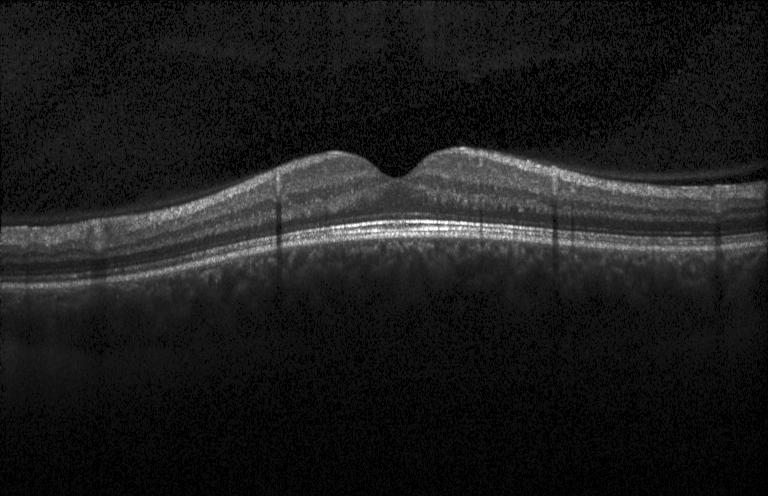

Retinal OCT B-scan
Dx: neither choroidal neovascularization, diabetic macular edema, nor drusen.